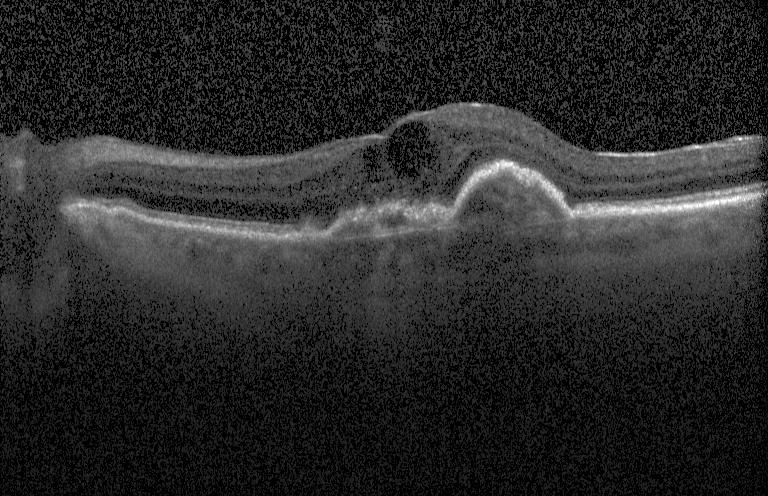 Optical coherence tomography B-scan.
The scan shows choroidal neovascularization.